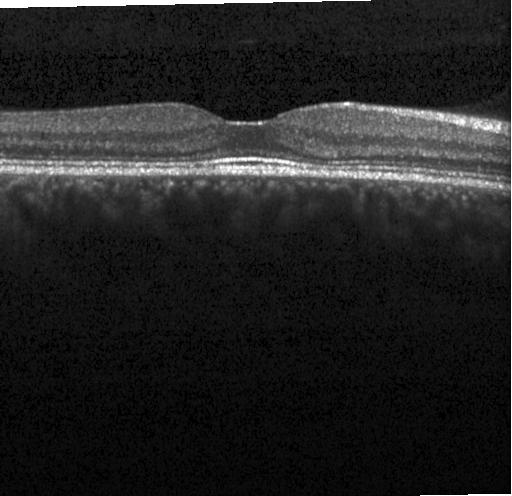 Optical coherence tomography scan — Assessment: no CNV, no DME, and no drusen.